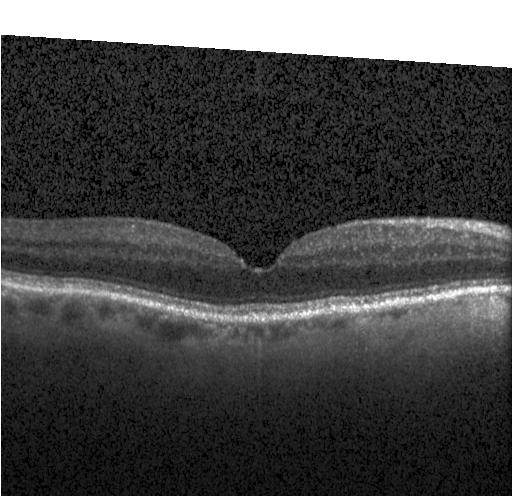

Retinal OCT B-scan — The scan shows no choroidal neovascularization, diabetic macular edema, or drusen.